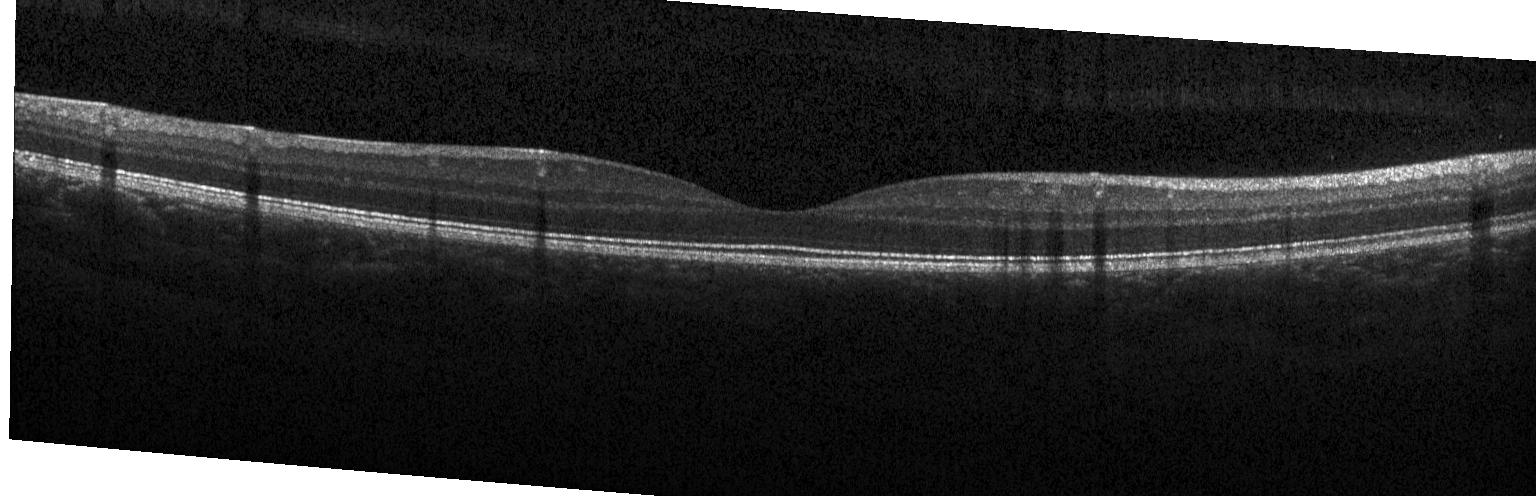 Diagnosis: neither choroidal neovascularization, diabetic macular edema, nor drusen.